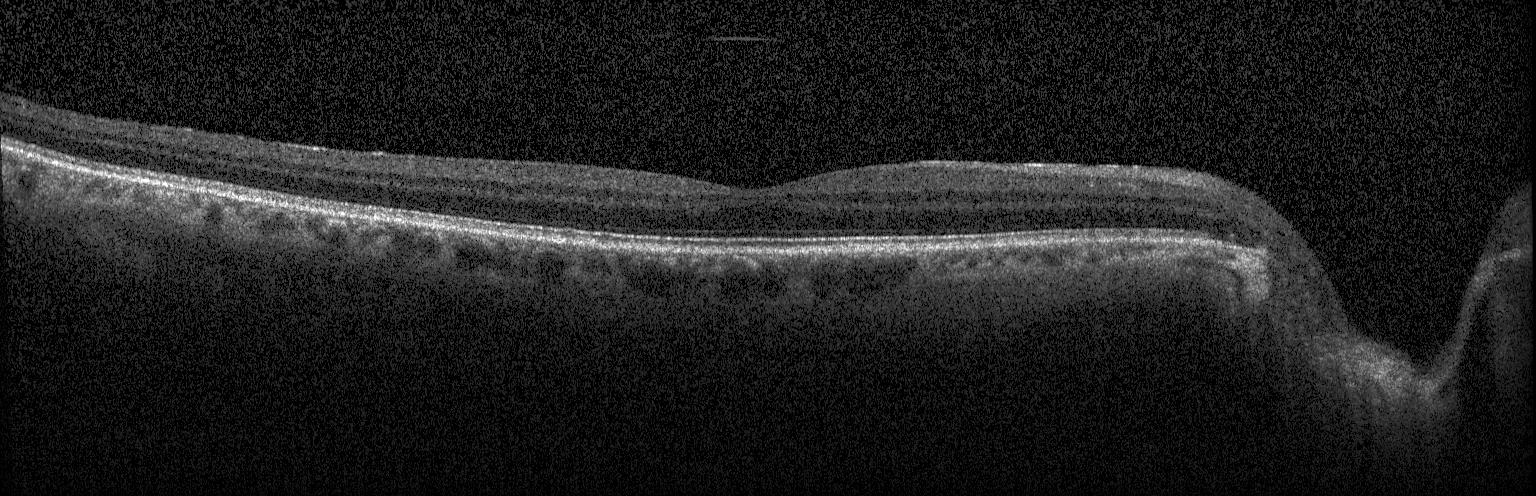

Retinal OCT cross-section showing no choroidal neovascularization, diabetic macular edema, or drusen.